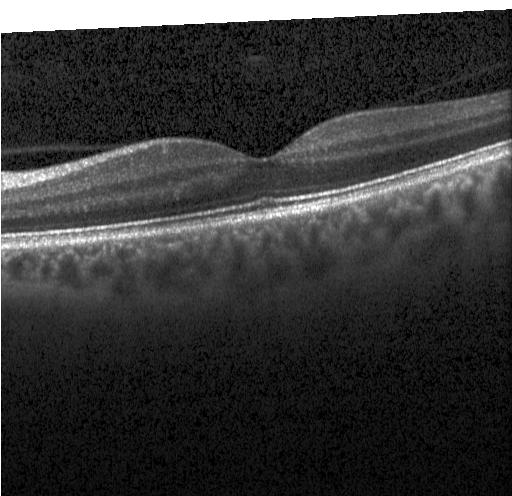

Optical coherence tomography scan.
This B-scan demonstrates no evidence of choroidal neovascularization, diabetic macular edema, or drusen.